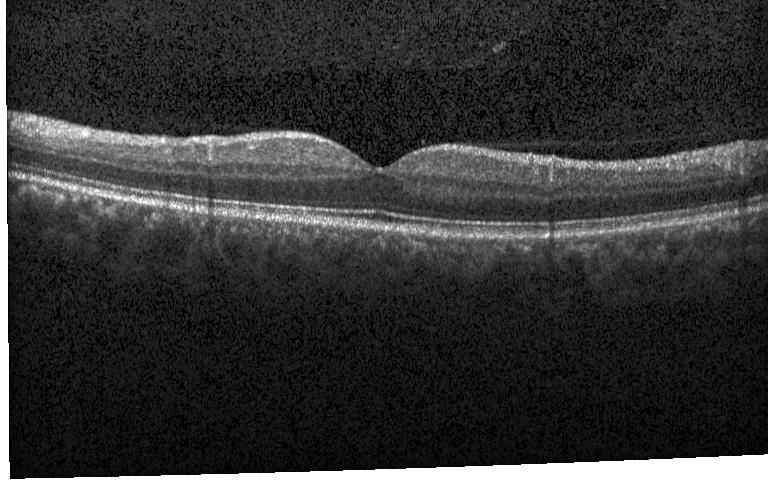 OCT line scan · through the macula · spectral-domain optical coherence tomography · Heidelberg Spectralis
Assessment: no evidence of choroidal neovascularization, diabetic macular edema, or drusen.